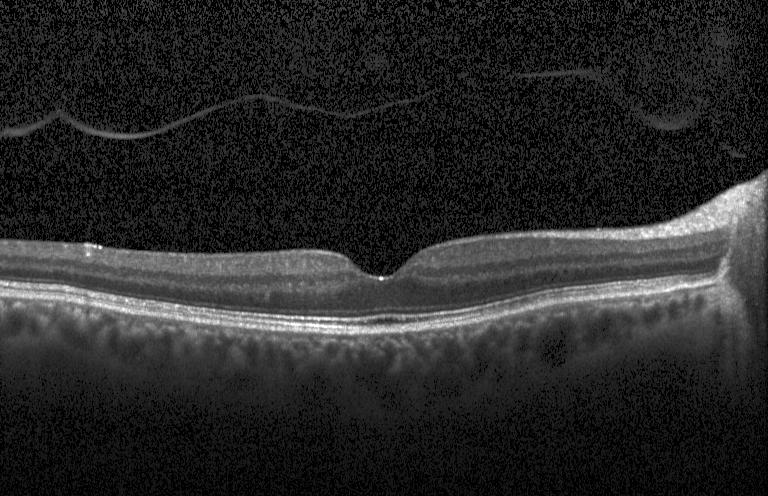

Retinal OCT cross-section
No evidence of choroidal neovascularization, diabetic macular edema, or drusen.